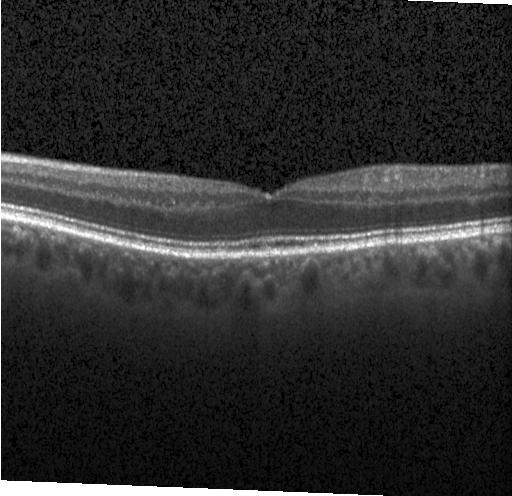
OCT line scan; macular scan
No choroidal neovascularization, diabetic macular edema, or drusen.